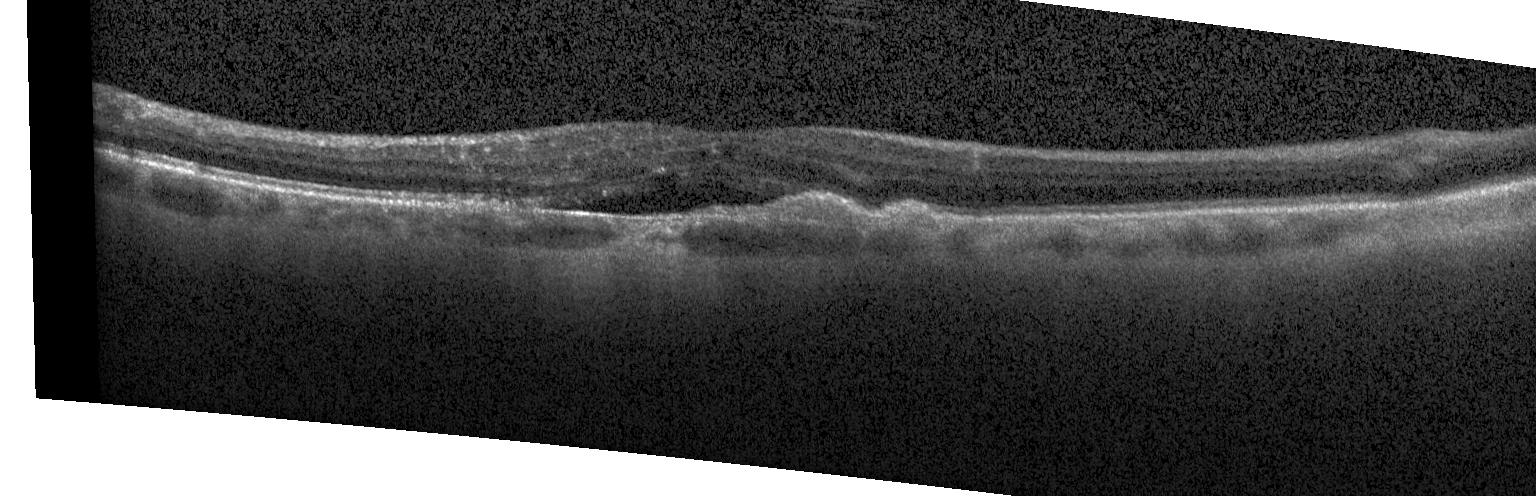
Macular OCT demonstrating a choroidal neovascular membrane.